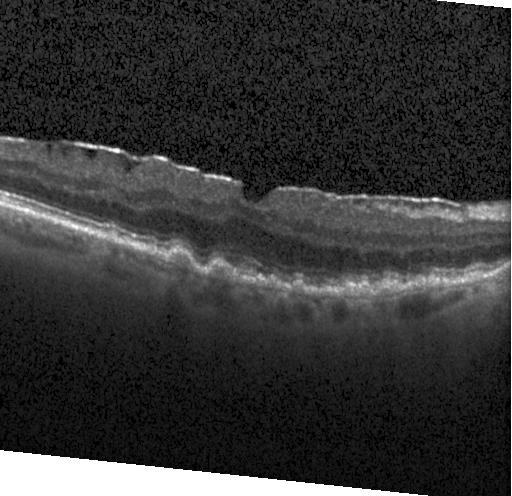

SD-OCT, retinal OCT B-scan
Finding: drusen.